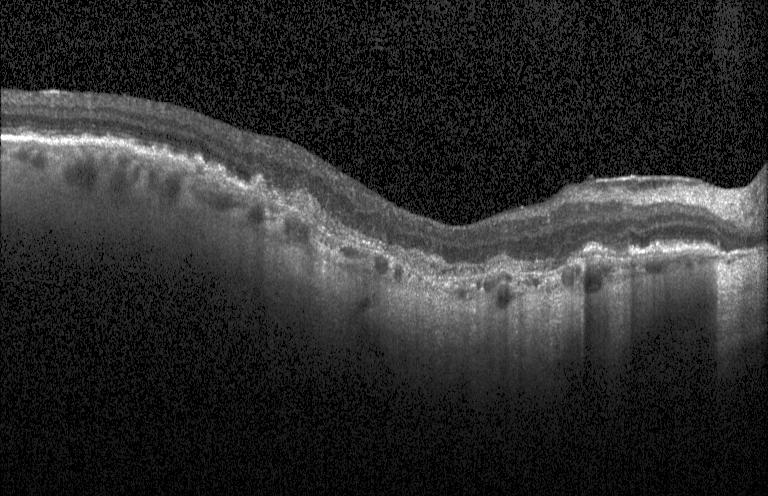 Finding: CNV.